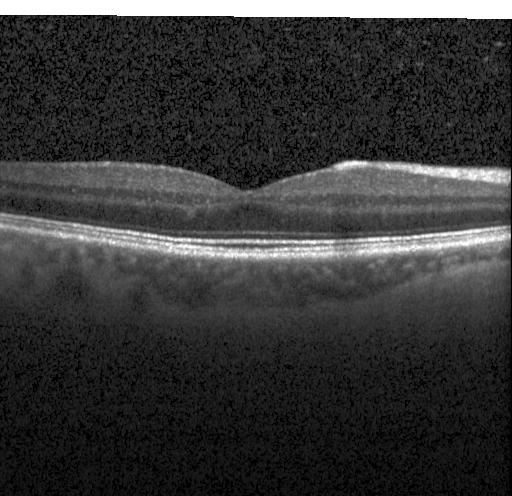 Optical coherence tomography scan.
Finding: no choroidal neovascularization, no diabetic macular edema, and no drusen.